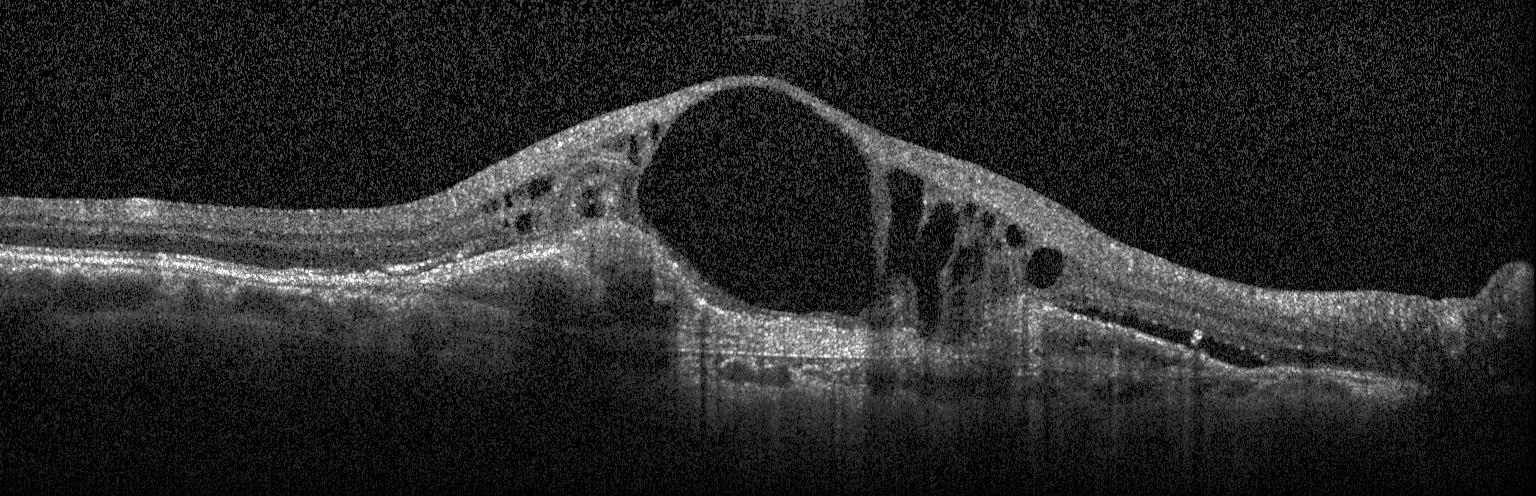 Fovea-centered, instrument: Heidelberg Spectralis, OCT B-scan — Assessment: a choroidal neovascular membrane.